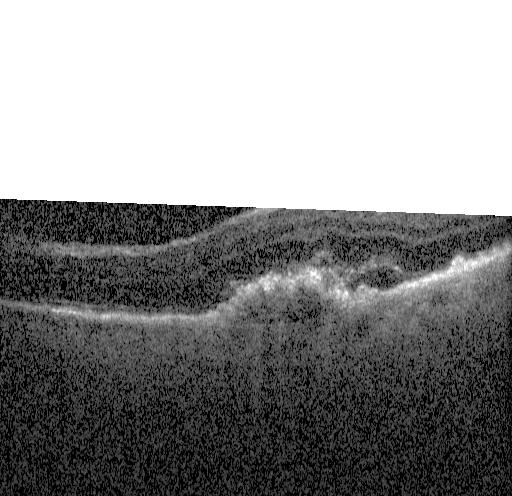 Impression: choroidal neovascularization (CNV).